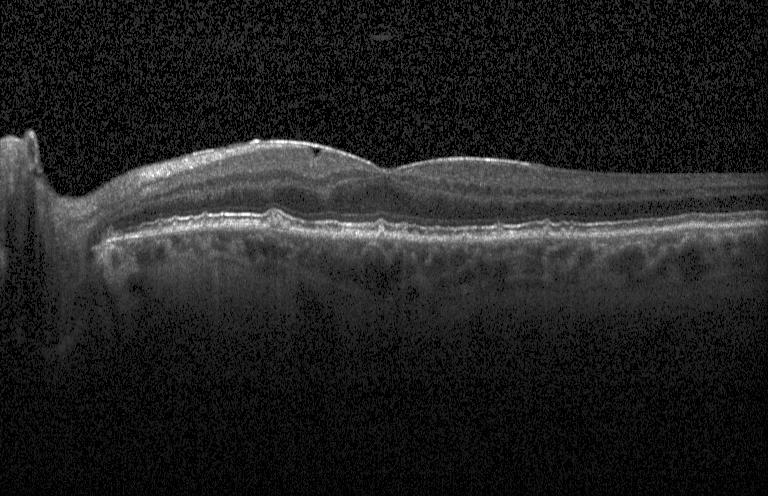 Heidelberg Spectralis. SD-OCT. Optical coherence tomography scan — Macular OCT: multiple drusen.